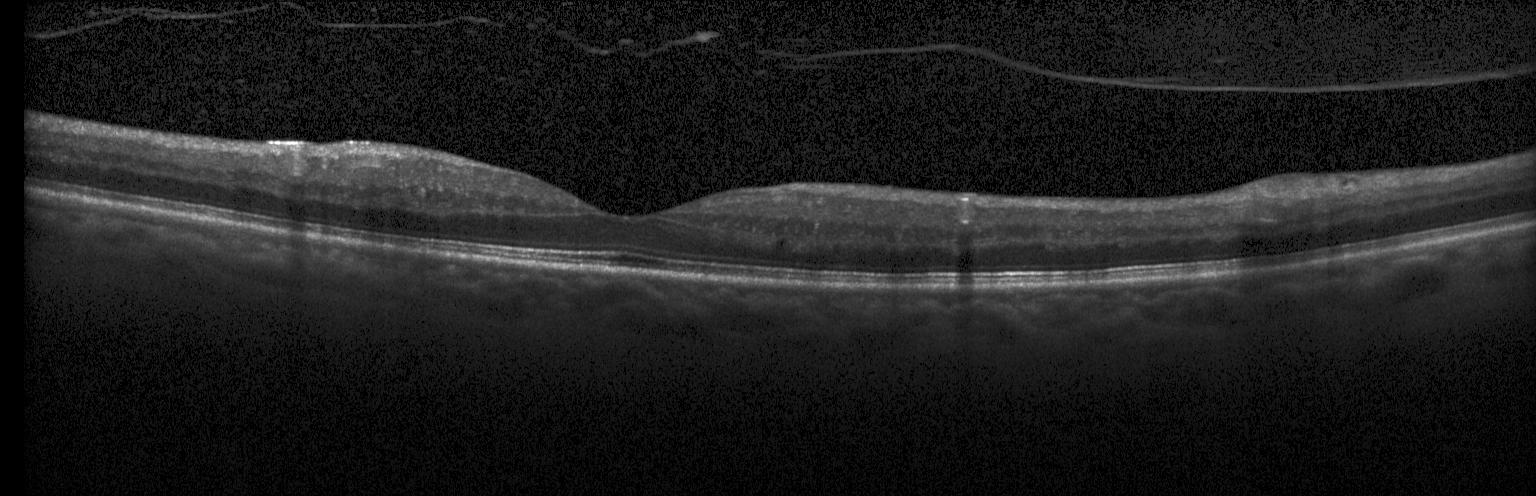 Spectral-domain optical coherence tomography, instrument: Heidelberg Spectralis, macular scan, OCT B-scan.
Diagnosis: no evidence of choroidal neovascularization, diabetic macular edema, or drusen.